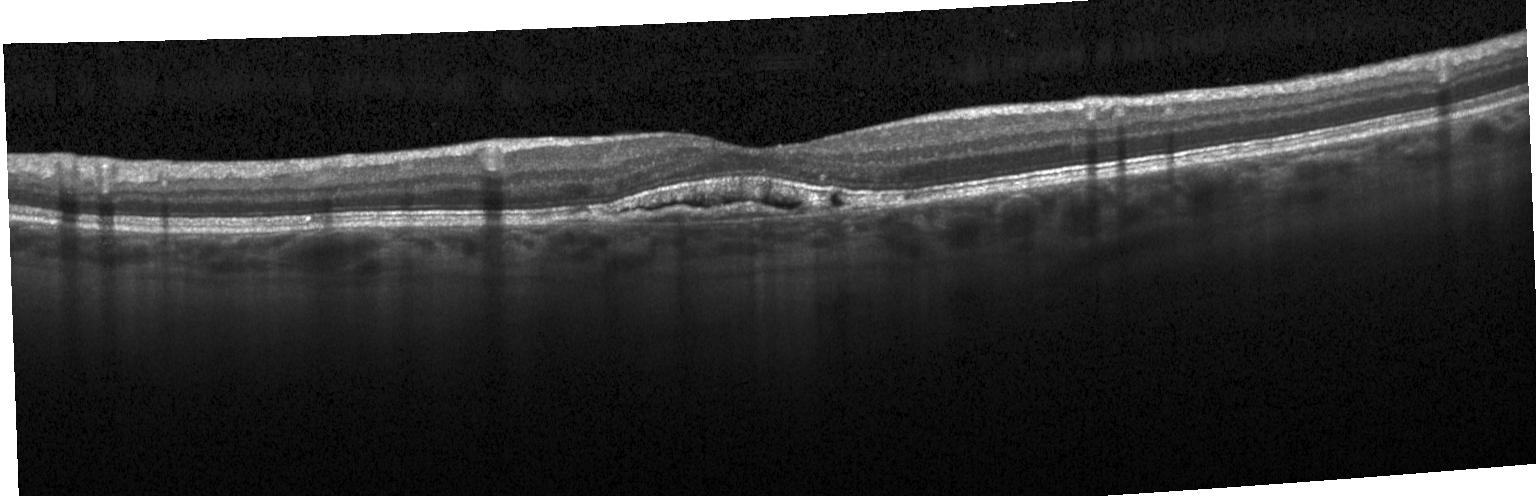
OCT B-scan
OCT finding: a choroidal neovascular membrane.